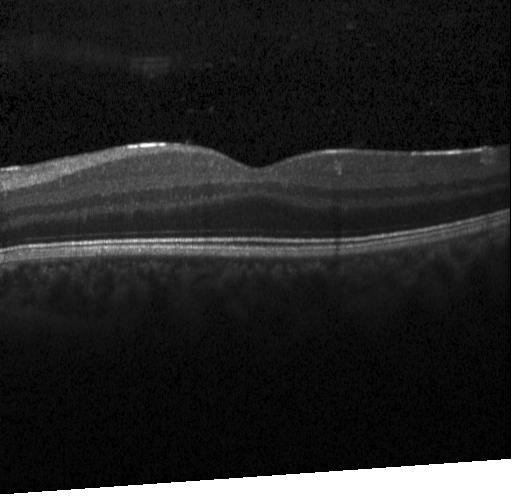

Optical coherence tomography B-scan, spectral-domain OCT. The scan shows no CNV, DME, or drusen.